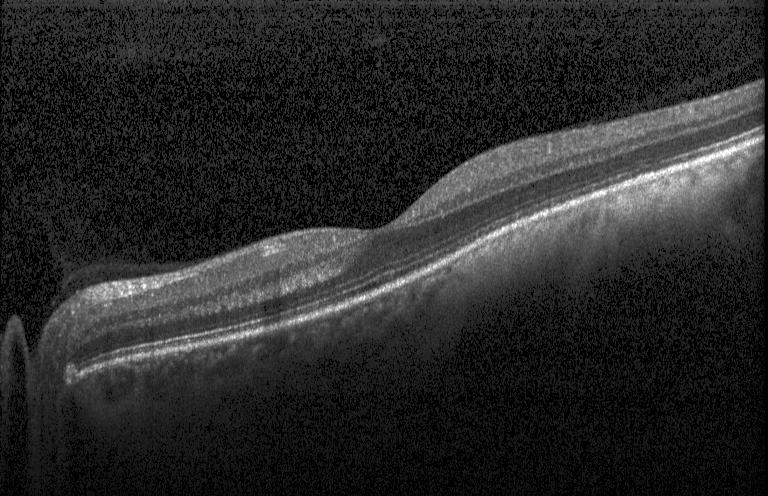
SD-OCT, Heidelberg Spectralis OCT system, through the macula, OCT line scan
Finding: no CNV, no DME, and no drusen.